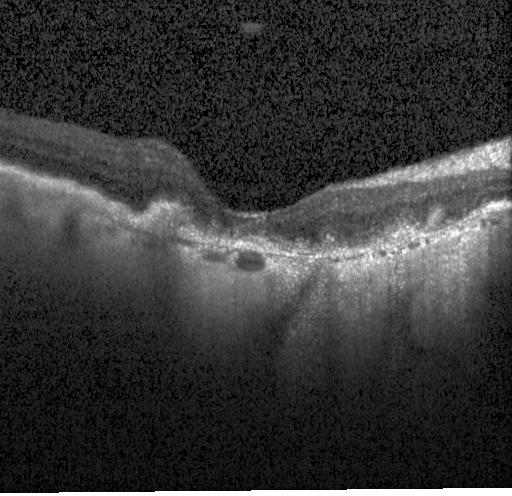

Spectral-domain optical coherence tomography. Fovea-centered. Heidelberg Spectralis OCT system. Optical coherence tomography scan
A choroidal neovascular membrane.